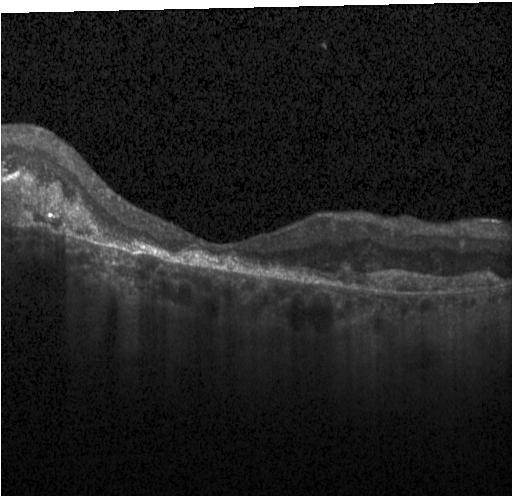 Spectral-domain optical coherence tomography · Heidelberg Spectralis · horizontal scan through the fovea · retinal OCT cross-section — Assessment: choroidal neovascularization.